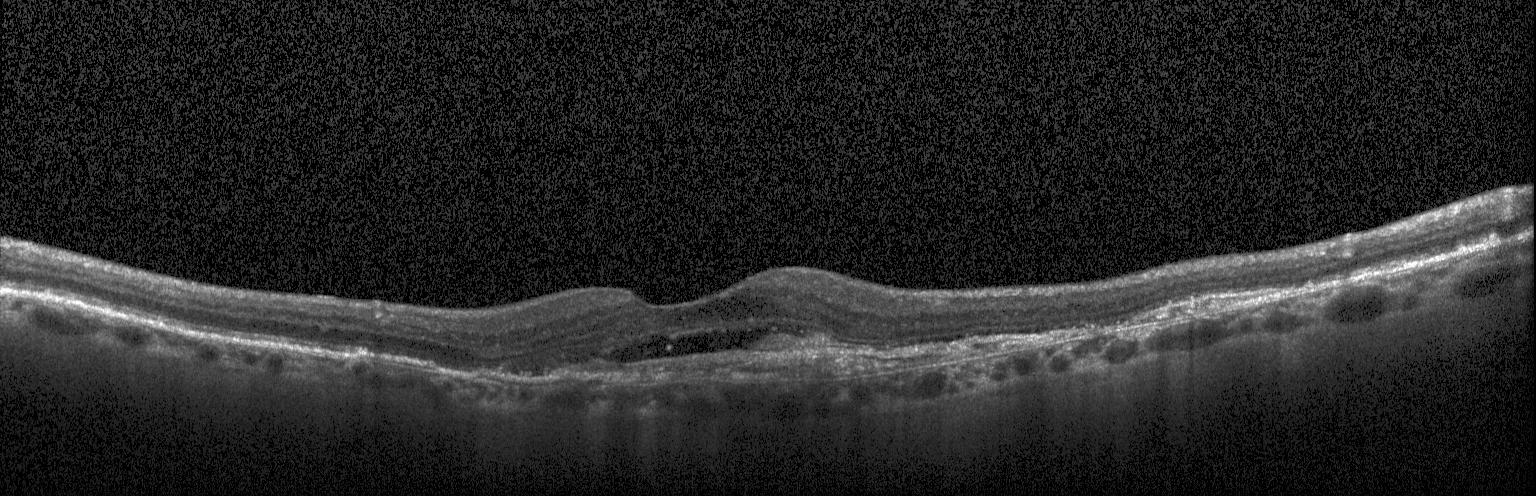

Optical coherence tomography scan.
Diagnosis: a choroidal neovascular membrane.